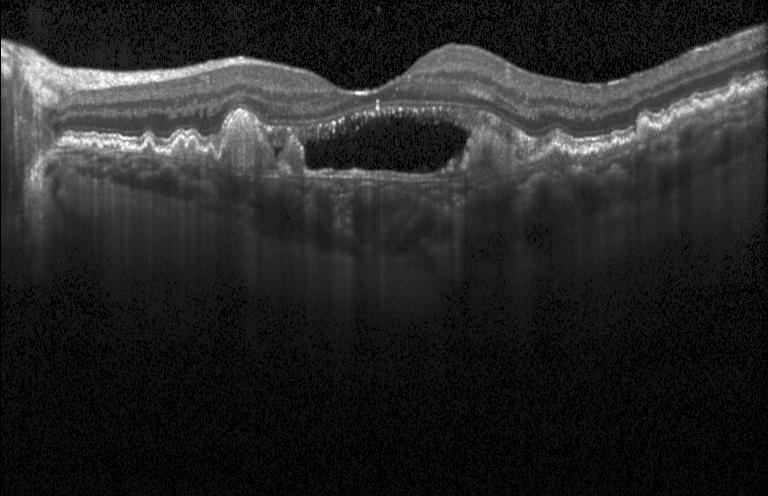 Impression: a choroidal neovascular membrane.